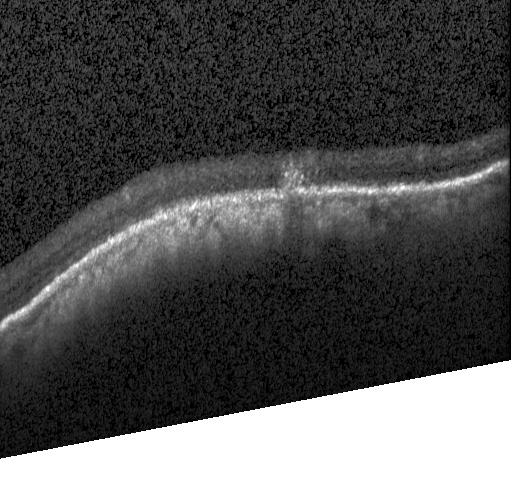

Macular OCT: a choroidal neovascular membrane.